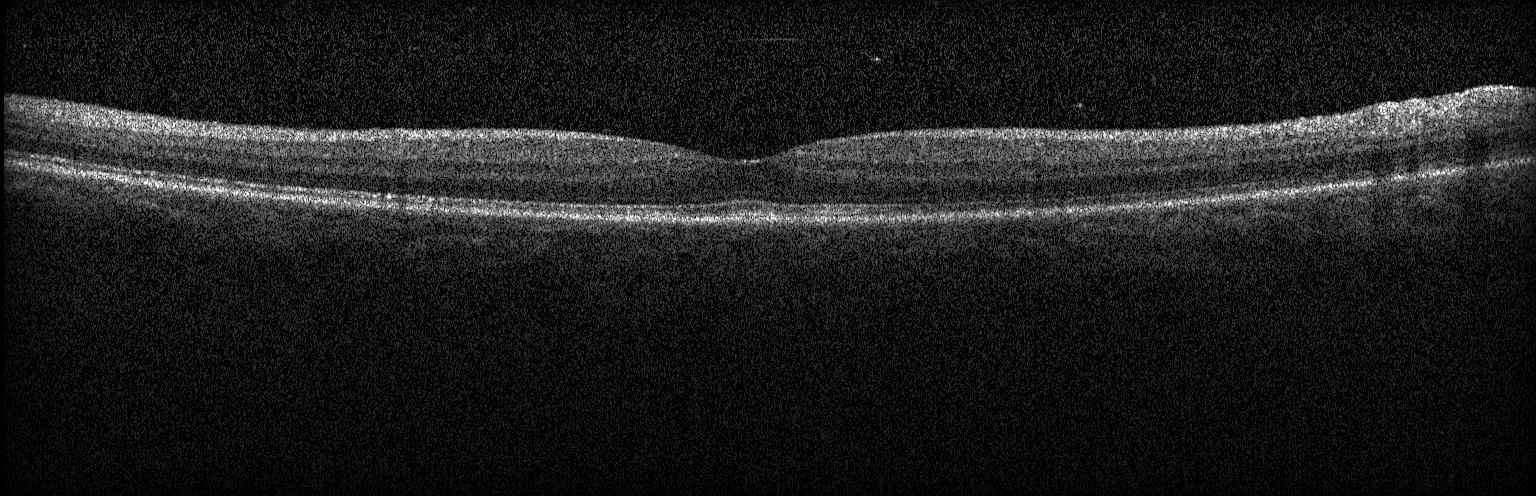 OCT B-scan showing no choroidal neovascularization, no diabetic macular edema, and no drusen.